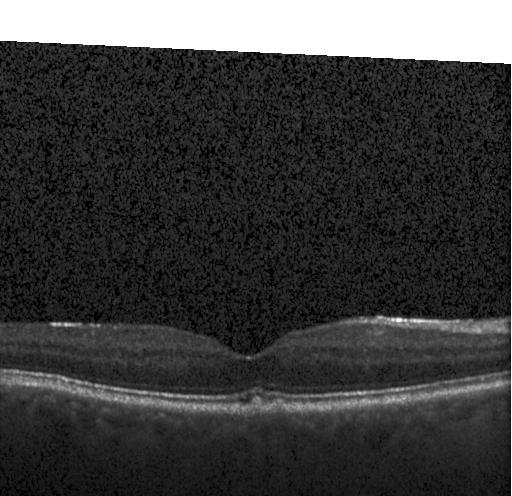
The scan shows drusen.